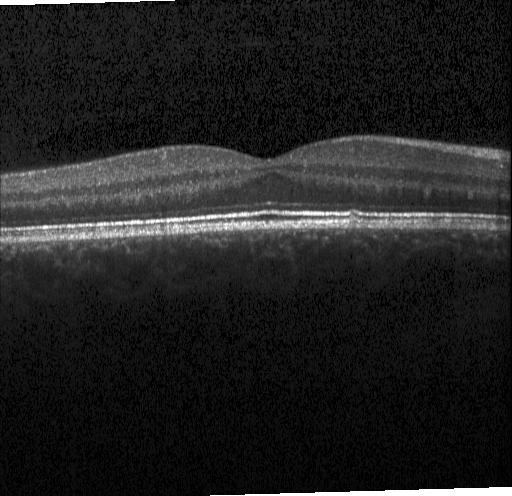
OCT finding: no choroidal neovascularization, diabetic macular edema, or drusen.